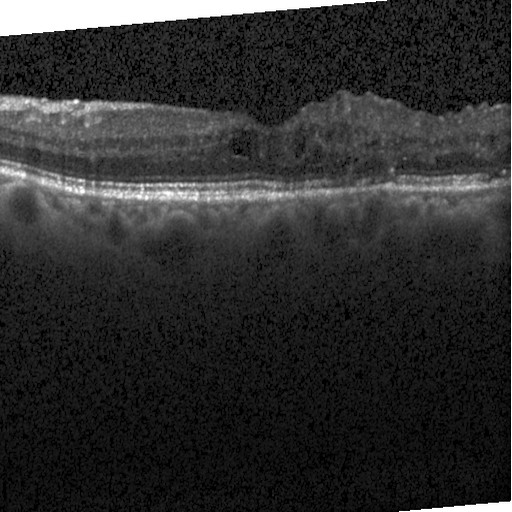 Horizontal scan through the fovea. OCT line scan — Diabetic macular edema.